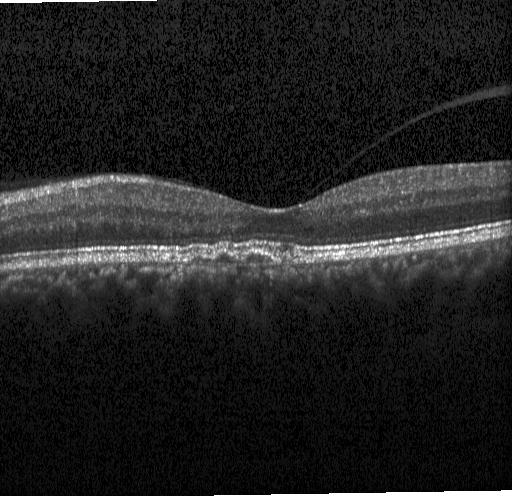
Spectral-domain OCT · acquired on a Heidelberg Spectralis · retinal OCT B-scan
Assessment: sub-RPE drusenoid deposits.